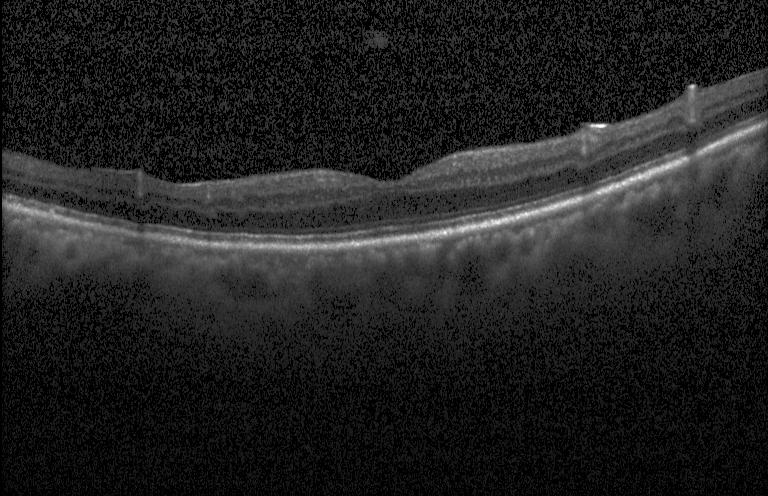 OCT B-scan. The scan shows no evidence of choroidal neovascularization, diabetic macular edema, or drusen.